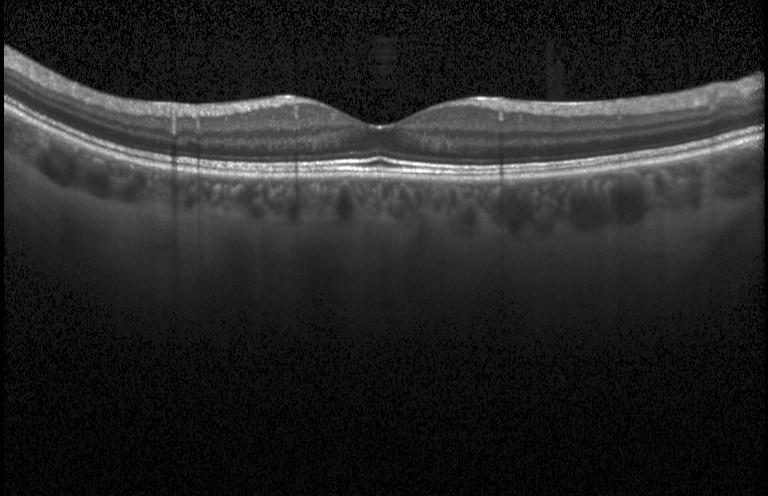

Retinal OCT cross-section; SD-OCT. Assessment: no evidence of choroidal neovascularization, diabetic macular edema, or drusen.